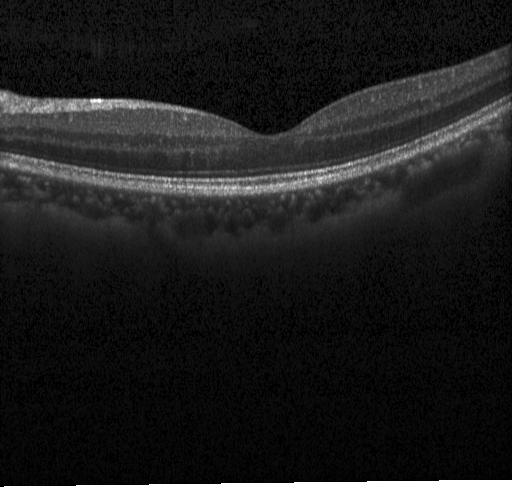
Heidelberg Spectralis OCT system · spectral-domain optical coherence tomography · OCT B-scan · macular scan.
Impression: neither choroidal neovascularization, diabetic macular edema, nor drusen.